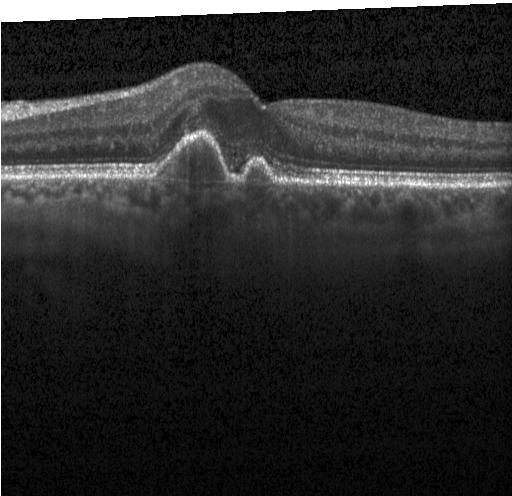 Macular OCT demonstrating choroidal neovascularization (CNV).